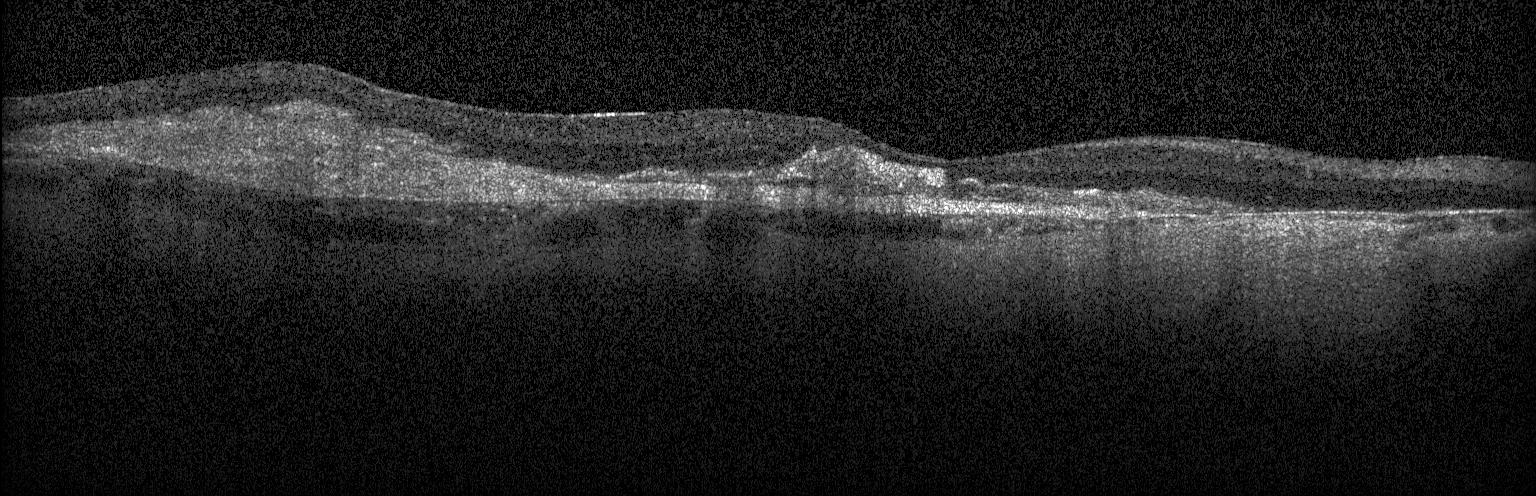
Spectral-domain OCT B-scan: a choroidal neovascular membrane.